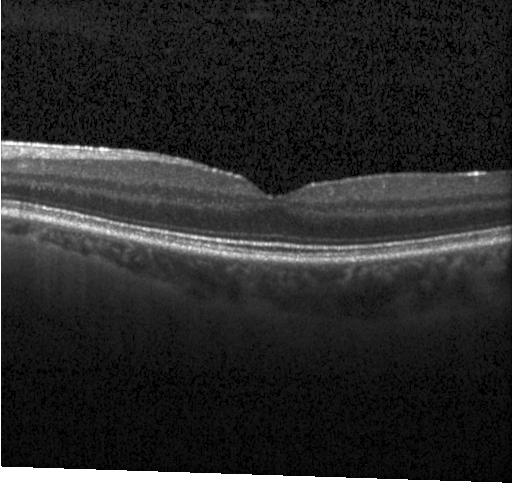

Instrument: Heidelberg Spectralis, spectral-domain optical coherence tomography, retinal OCT B-scan, horizontal scan through the fovea
Assessment: neither CNV, DME, nor drusen.